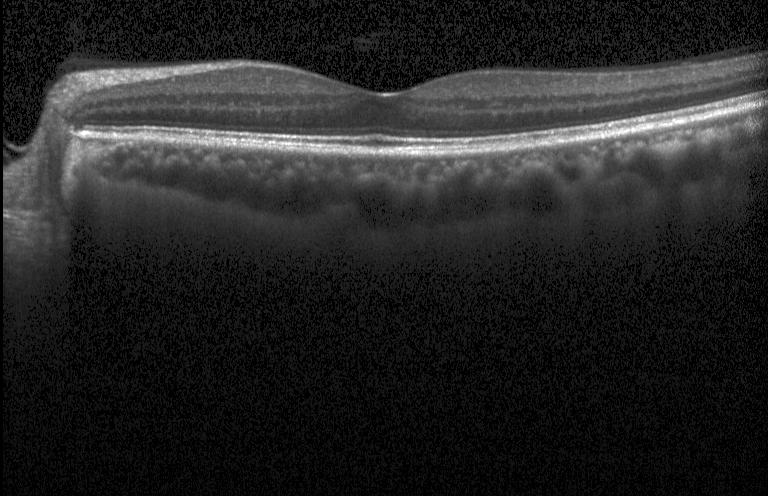
Finding: neither CNV, DME, nor drusen.